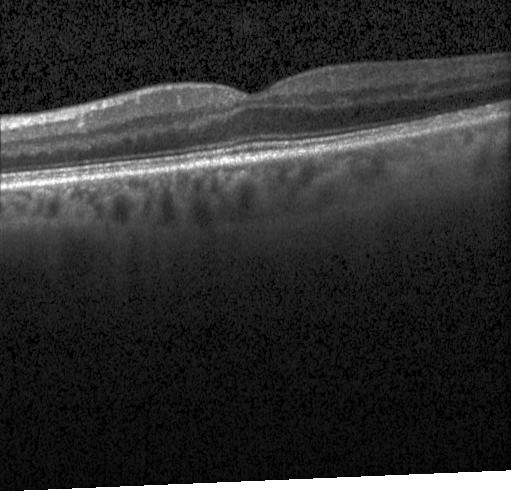
Macular scan; OCT B-scan; acquired on a Heidelberg Spectralis — Diagnosis: neither choroidal neovascularization, diabetic macular edema, nor drusen.